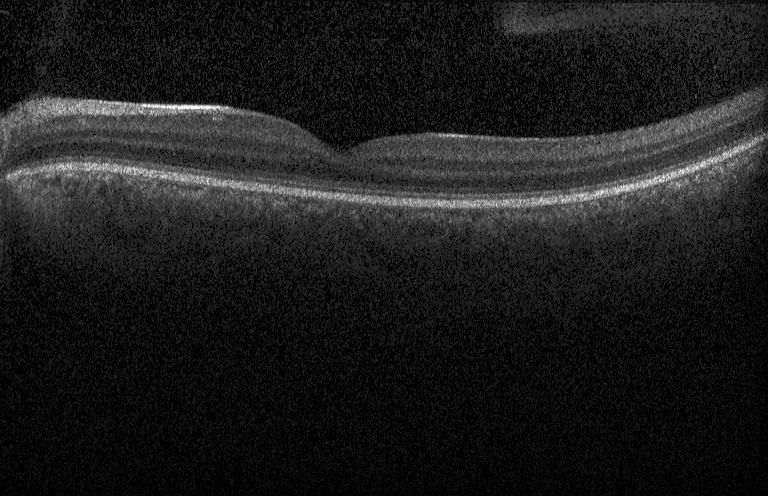
OCT B-scan.
Impression: no choroidal neovascularization, diabetic macular edema, or drusen.